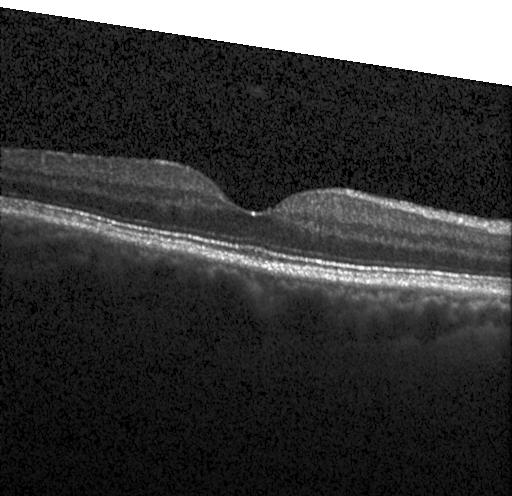 SD-OCT, instrument: Heidelberg Spectralis, optical coherence tomography B-scan — This B-scan demonstrates no choroidal neovascularization, no diabetic macular edema, and no drusen.